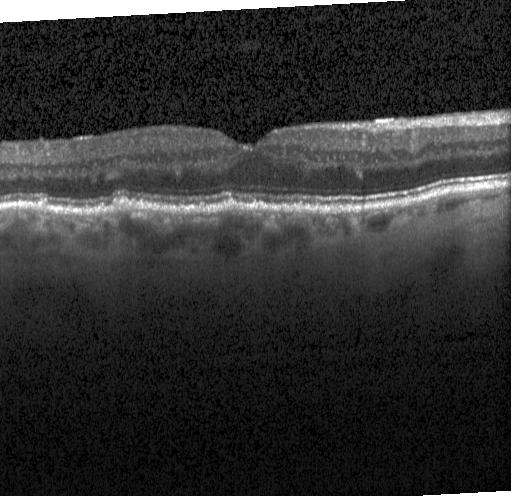 Optical coherence tomography B-scan. The scan shows multiple drusen.